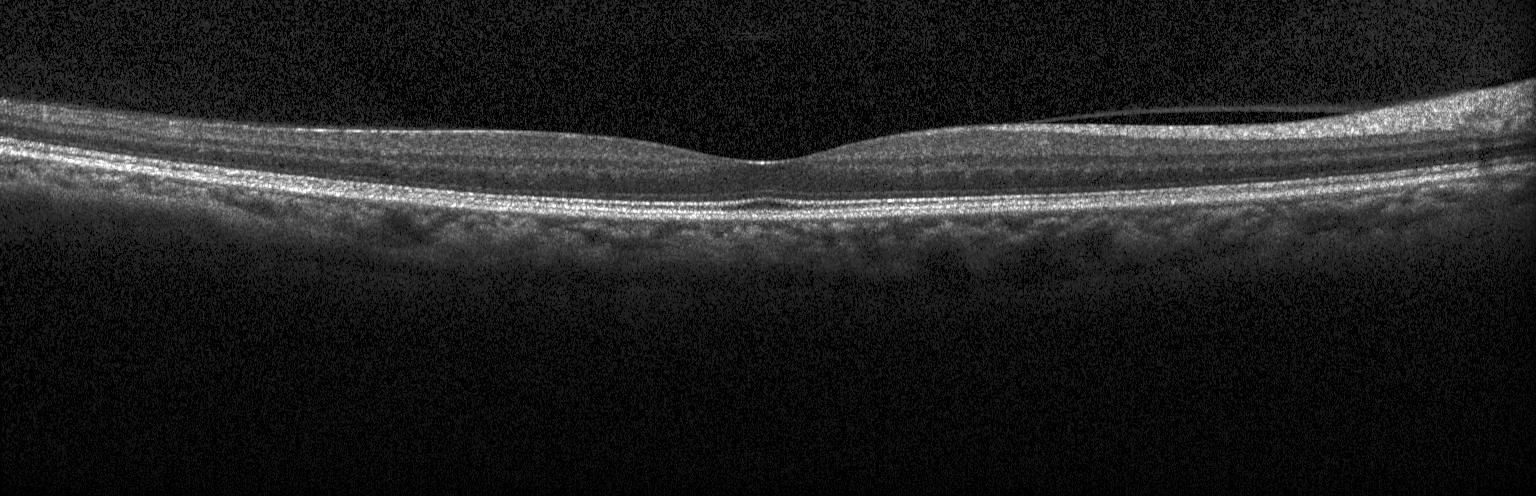
Centered on the fovea, optical coherence tomography B-scan.
Finding: neither choroidal neovascularization, diabetic macular edema, nor drusen.